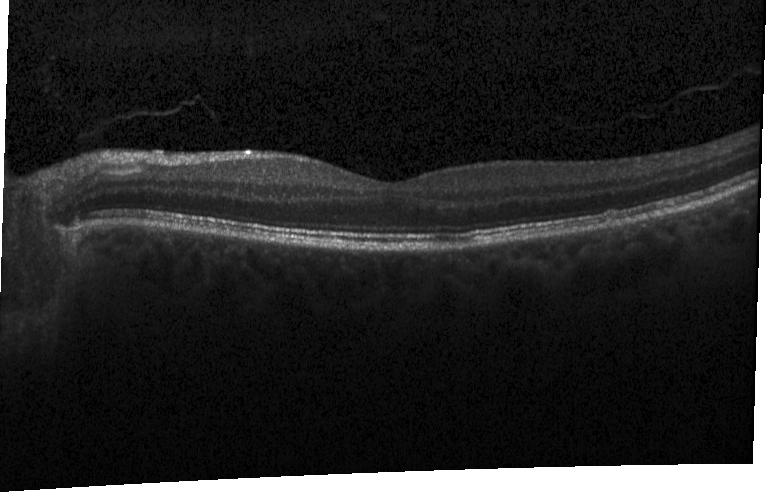

OCT B-scan
Diagnosis: no CNV, DME, or drusen.